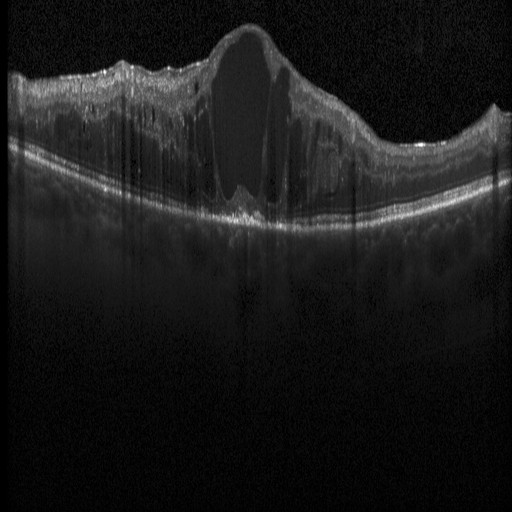 Macular OCT: diabetic macular edema.